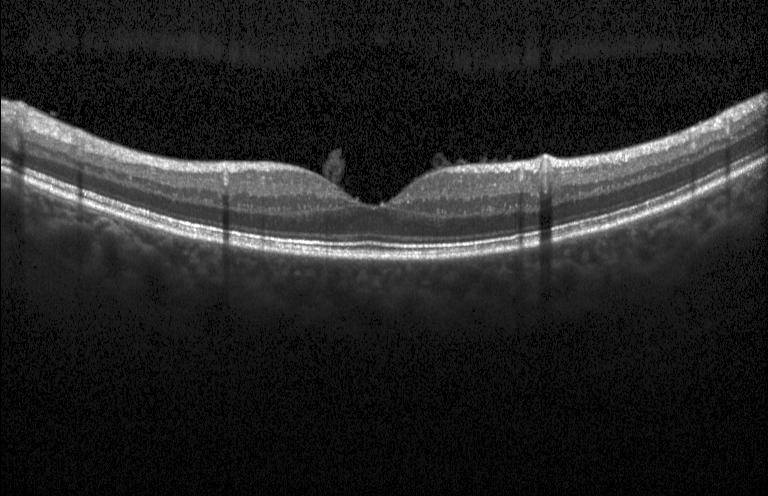
Diagnosis: no choroidal neovascularization, no diabetic macular edema, and no drusen.